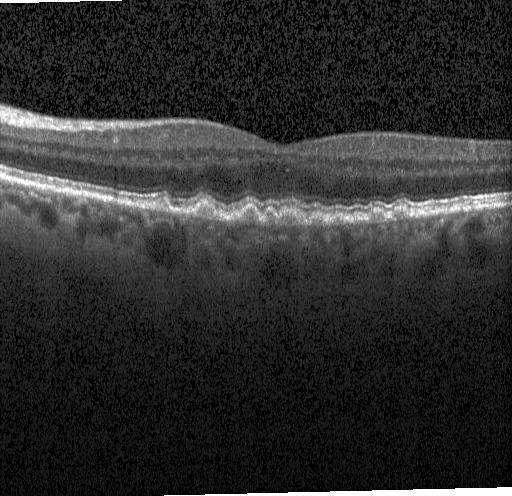
Impression: drusen.